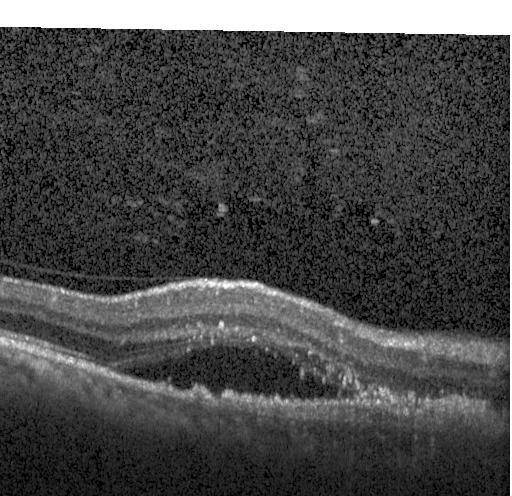
Finding: a choroidal neovascular membrane.